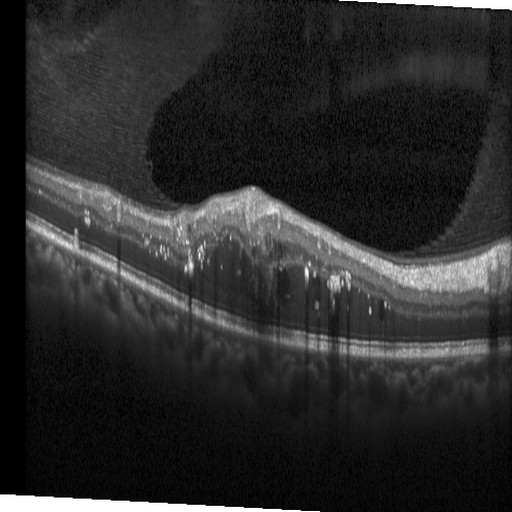
Spectral-domain OCT B-scan: DME.